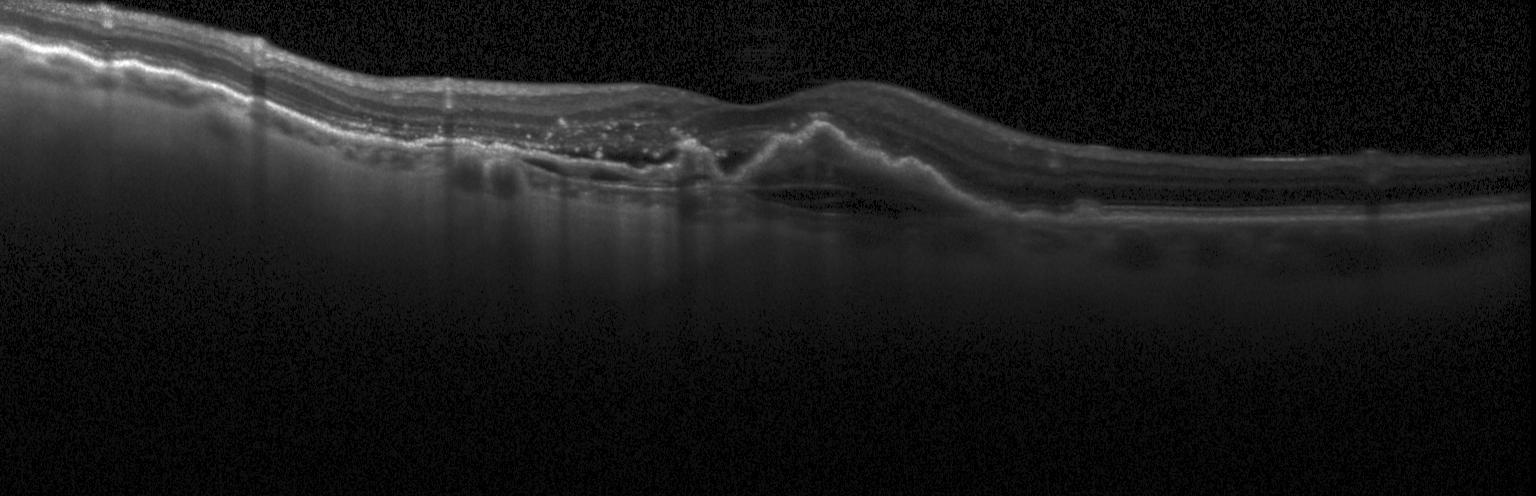
Heidelberg Spectralis. Optical coherence tomography B-scan.
Dx: a choroidal neovascular membrane.